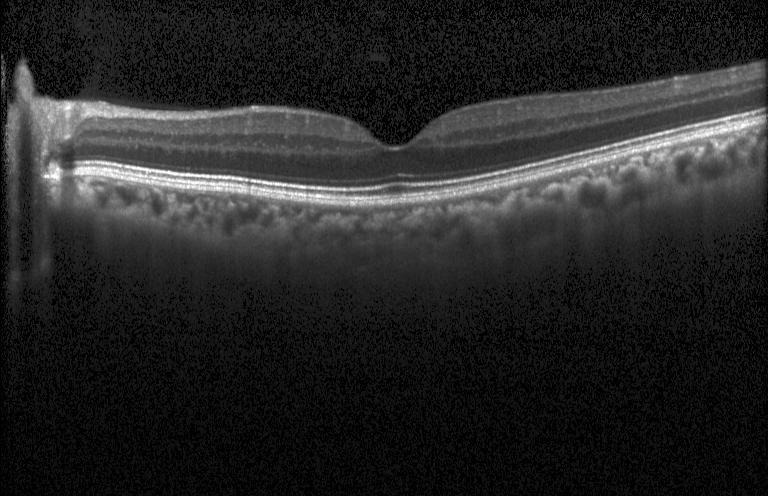 Macular OCT: no CNV, no DME, and no drusen.